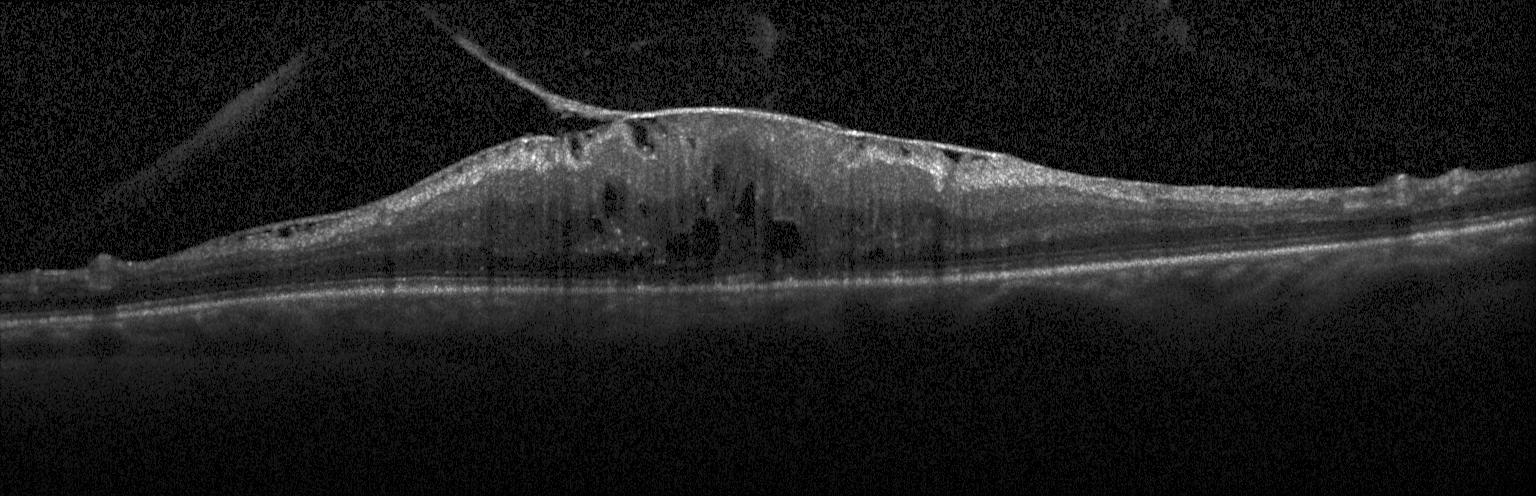 This B-scan demonstrates DME.